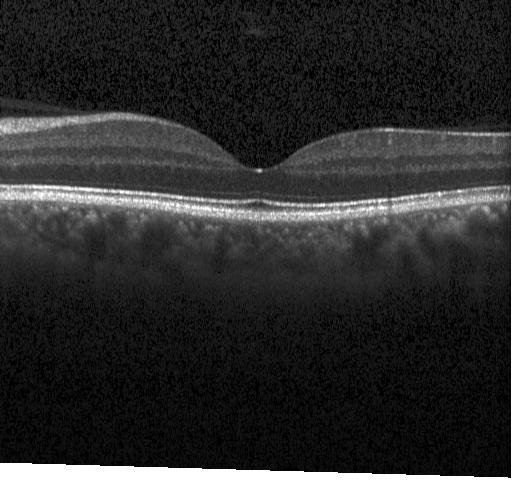 Through the macula. Retinal OCT B-scan. SD-OCT
Assessment: no choroidal neovascularization, no diabetic macular edema, and no drusen.